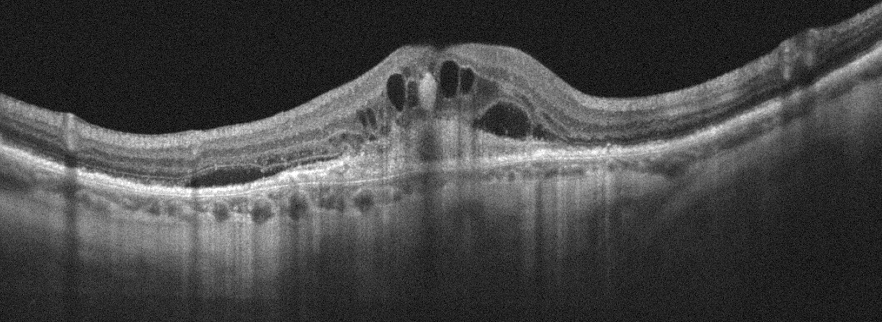 OCT B-scan, oculus dexter.
Impression: age-related macular degeneration (AMD).